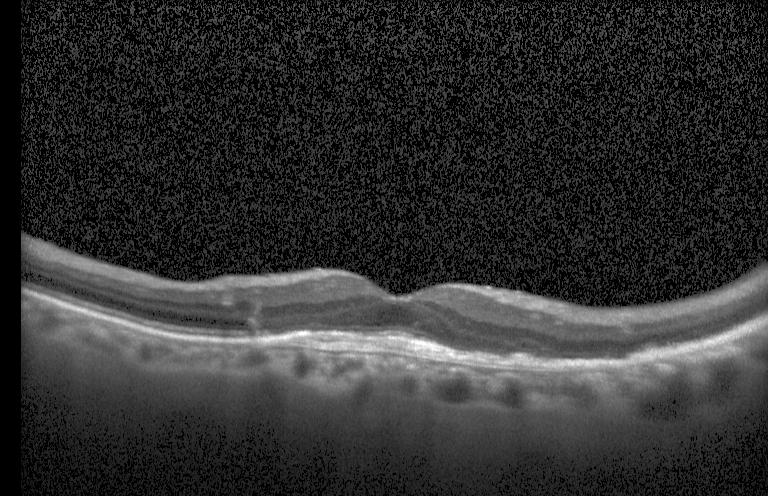
Heidelberg Spectralis. Retinal OCT B-scan. SD-OCT
Impression: a choroidal neovascular membrane.